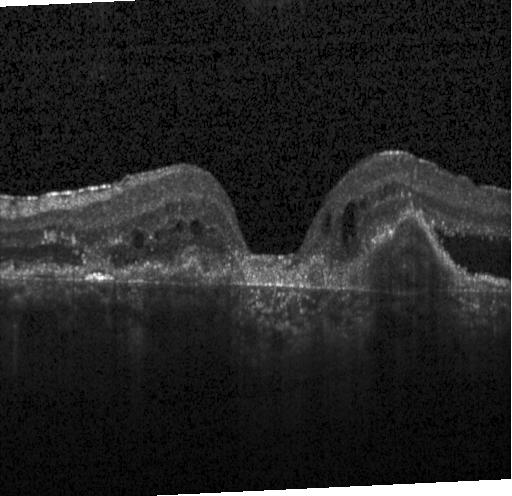

Optical coherence tomography B-scan. SD-OCT. Heidelberg Spectralis OCT system
Impression: a choroidal neovascular membrane.